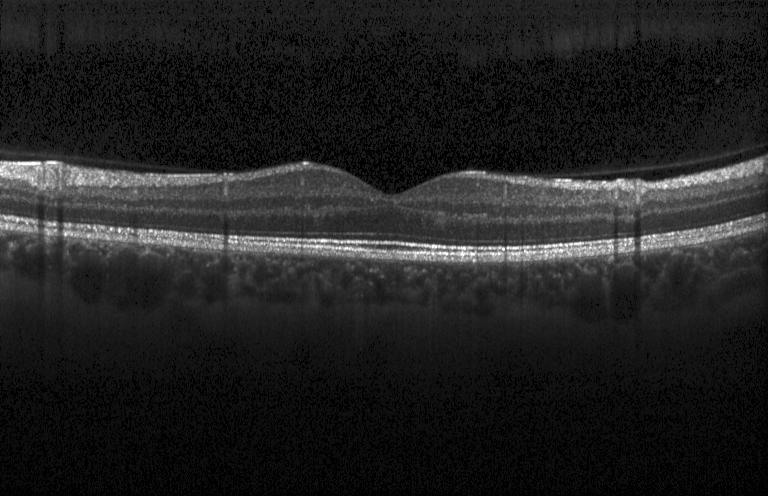 Retinal OCT cross-section — Finding: neither CNV, DME, nor drusen.